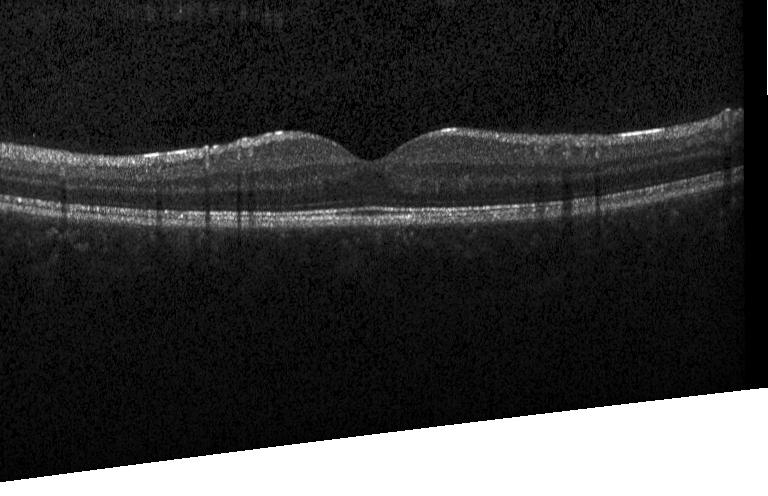

No evidence of choroidal neovascularization, diabetic macular edema, or drusen.